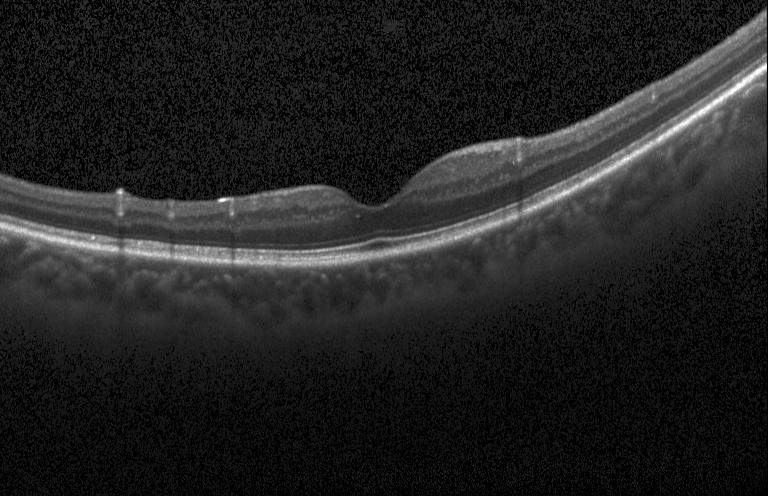

Assessment: neither CNV, DME, nor drusen.